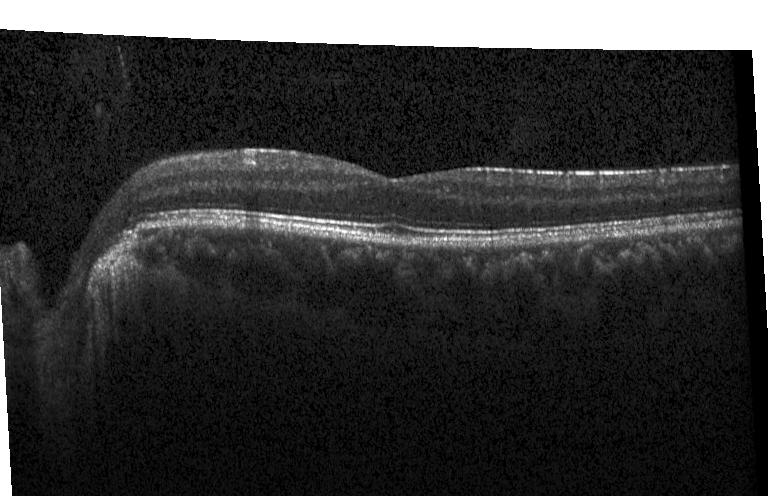 Optical coherence tomography scan, SD-OCT, through the macula, acquired on a Heidelberg Spectralis. Macular OCT: no evidence of CNV, DME, or drusen.